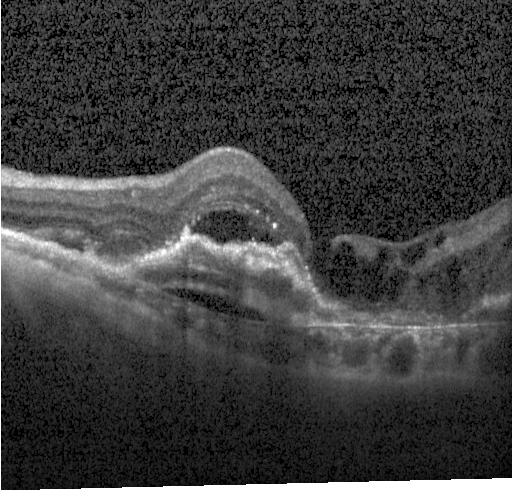 This B-scan demonstrates CNV.